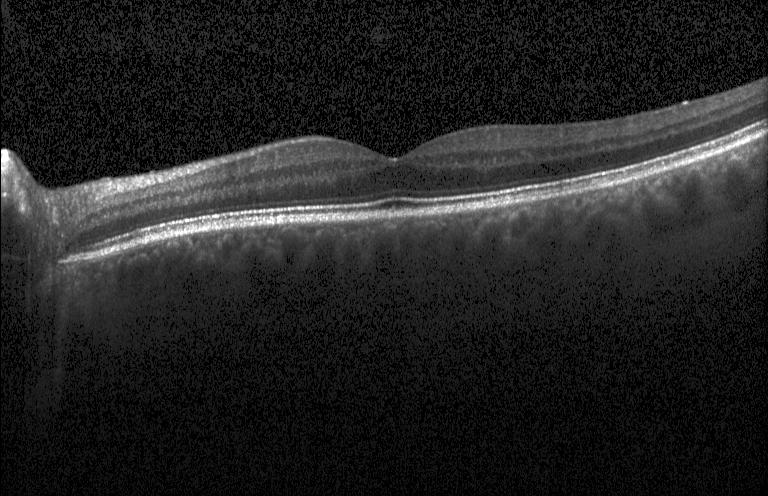
Fovea-centered; SD-OCT; OCT line scan — Macular OCT: no choroidal neovascularization, diabetic macular edema, or drusen.